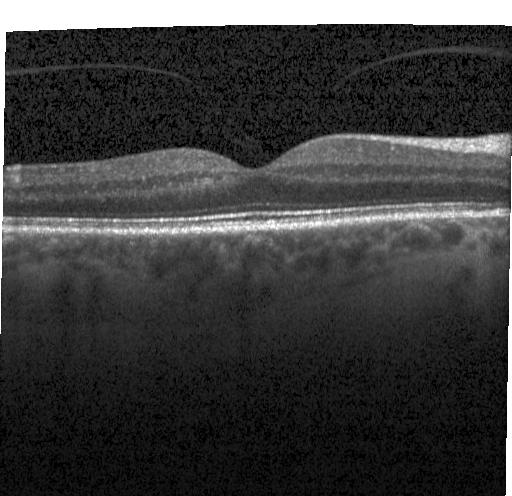

Finding: no evidence of choroidal neovascularization, diabetic macular edema, or drusen.